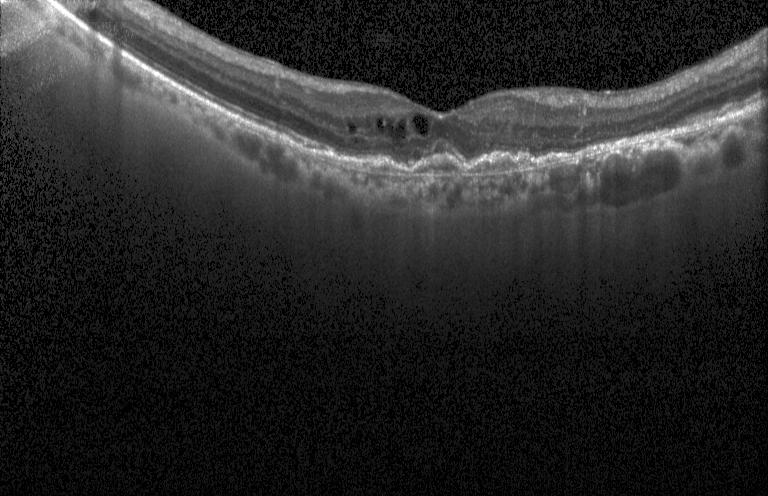

This B-scan demonstrates a choroidal neovascular membrane.